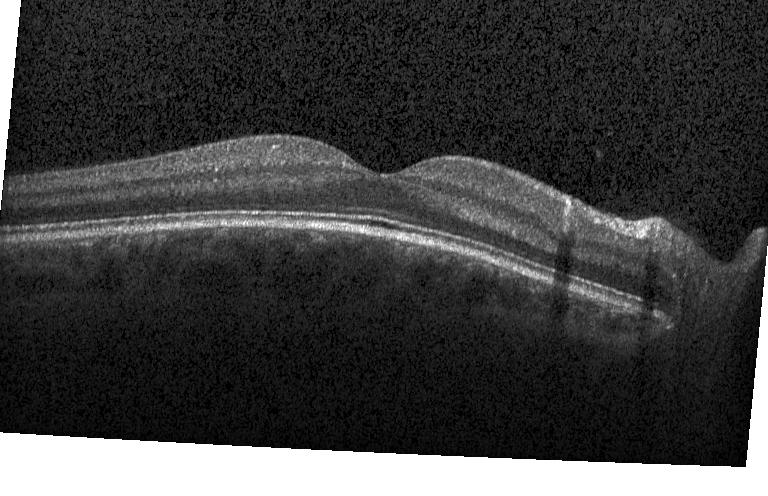 Optical coherence tomography B-scan, Heidelberg Spectralis OCT system
This B-scan demonstrates no choroidal neovascularization, no diabetic macular edema, and no drusen.